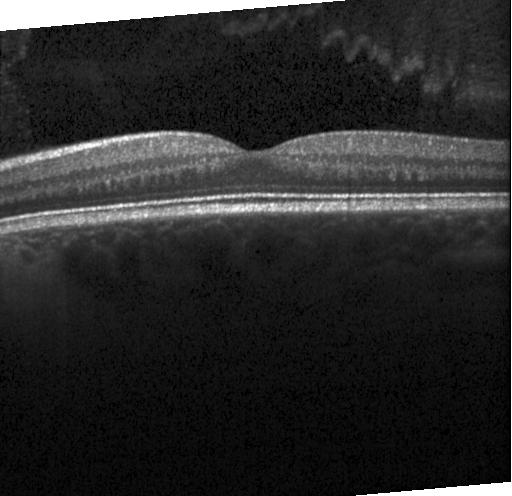
OCT B-scan showing no choroidal neovascularization, no diabetic macular edema, and no drusen.